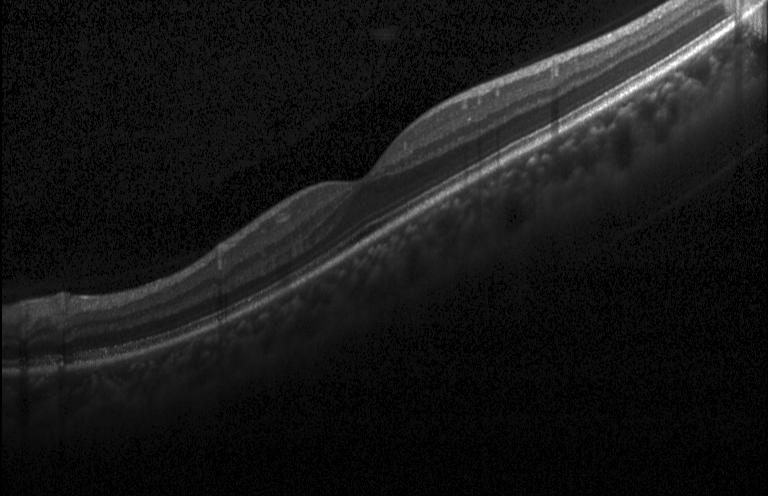 Horizontal scan through the fovea; Heidelberg Spectralis OCT system; optical coherence tomography scan — No evidence of choroidal neovascularization, diabetic macular edema, or drusen.